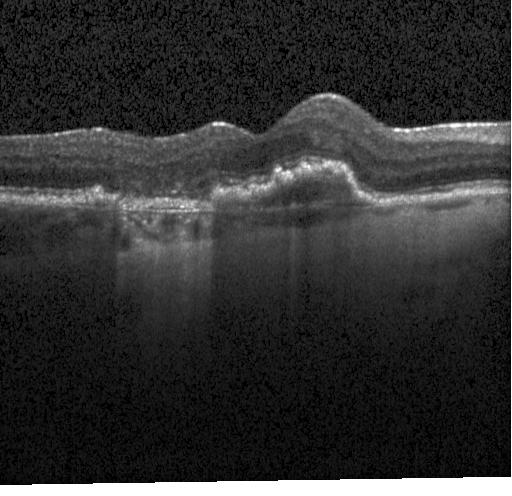 Through the macula, Heidelberg Spectralis OCT system, SD-OCT, OCT B-scan — The scan shows a choroidal neovascular membrane.